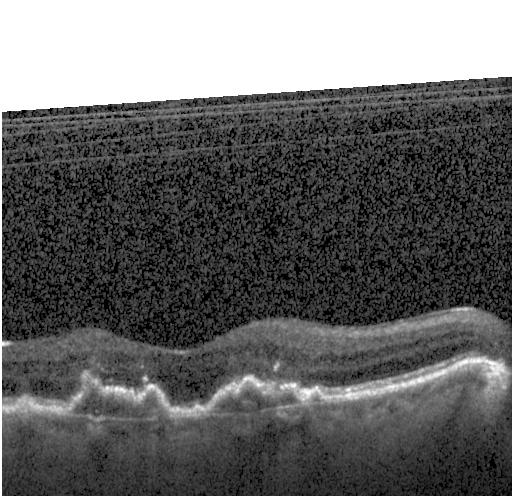

Macular scan; optical coherence tomography scan; spectral-domain optical coherence tomography; instrument: Heidelberg Spectralis. Diagnosis: a choroidal neovascular membrane.